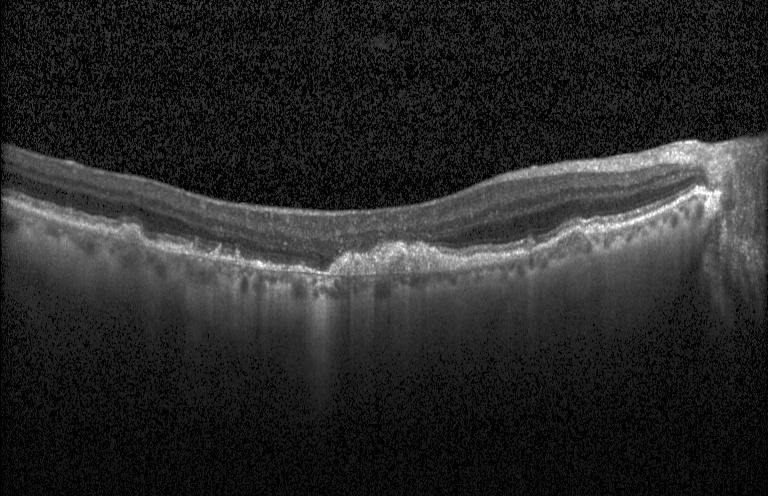 Assessment: choroidal neovascularization.